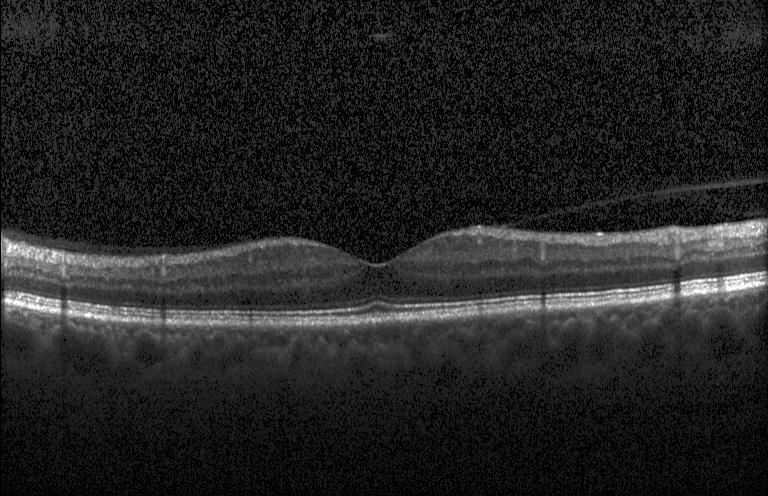

Retinal OCT cross-section showing no CNV, DME, or drusen.